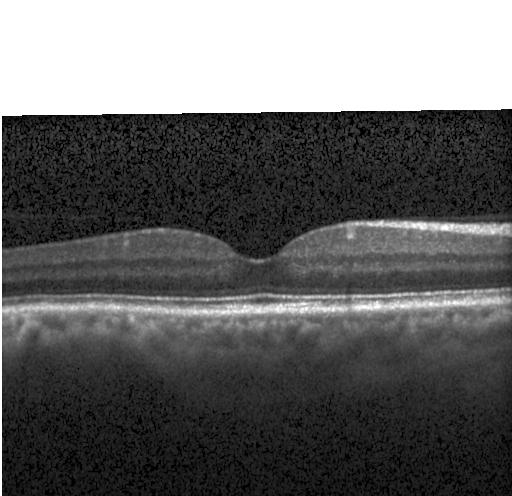 Assessment: neither choroidal neovascularization, diabetic macular edema, nor drusen.